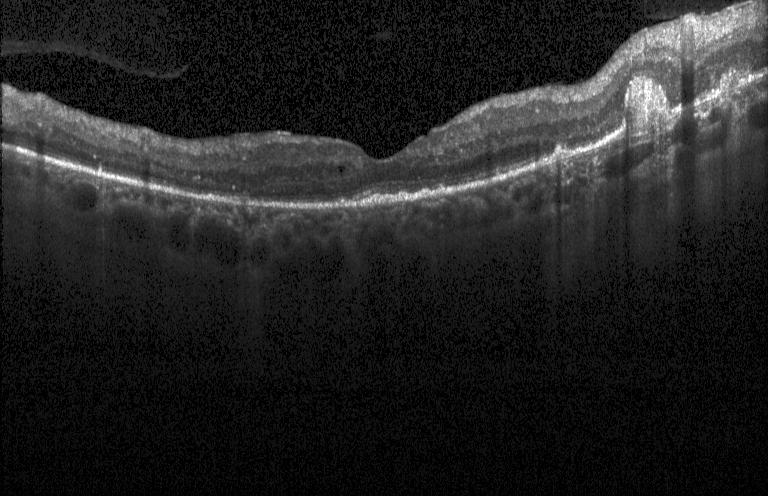
Optical coherence tomography scan; instrument: Heidelberg Spectralis
Impression: choroidal neovascularization (CNV).